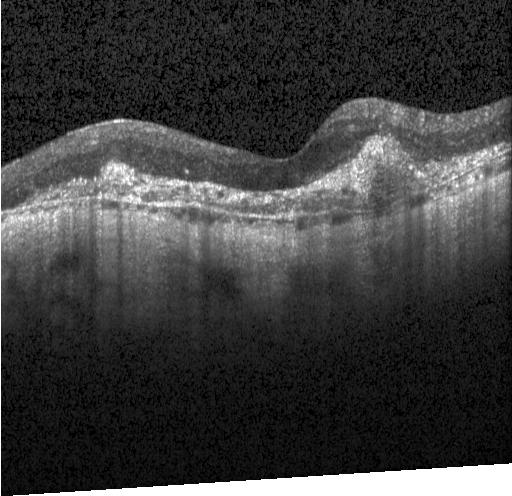

OCT B-scan · acquired on a Heidelberg Spectralis · SD-OCT
Diagnosis: choroidal neovascularization.